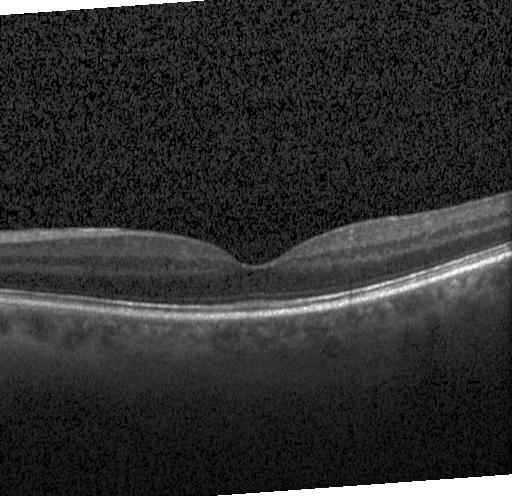 Retinal OCT cross-section — No choroidal neovascularization, diabetic macular edema, or drusen.